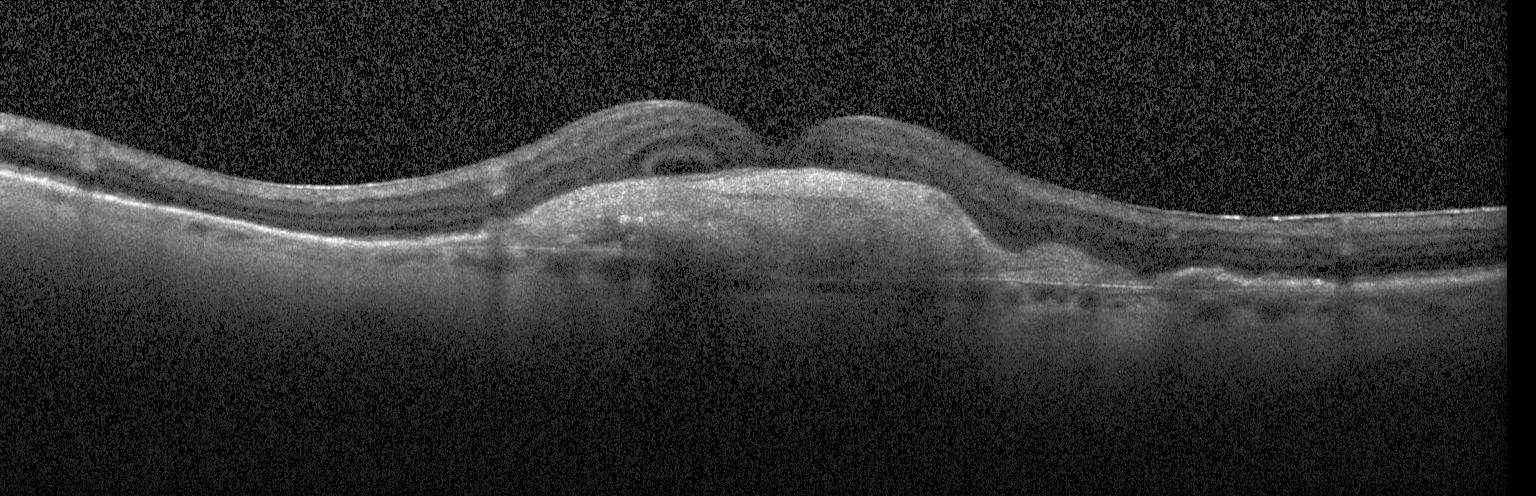

Choroidal neovascularization (CNV).